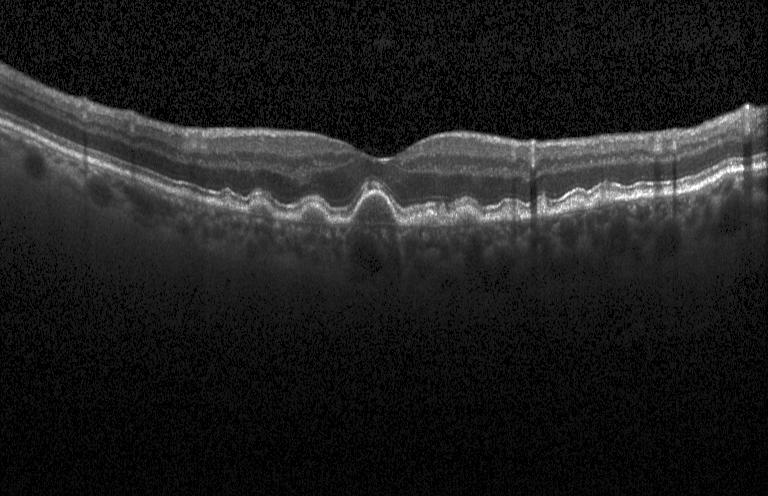

Spectral-domain optical coherence tomography. OCT line scan. Macular scan. Instrument: Heidelberg Spectralis
OCT finding: sub-RPE drusenoid deposits.